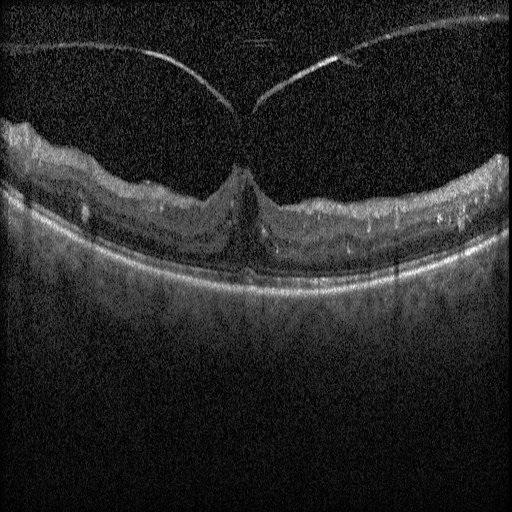

OCT finding: diabetic macular edema.